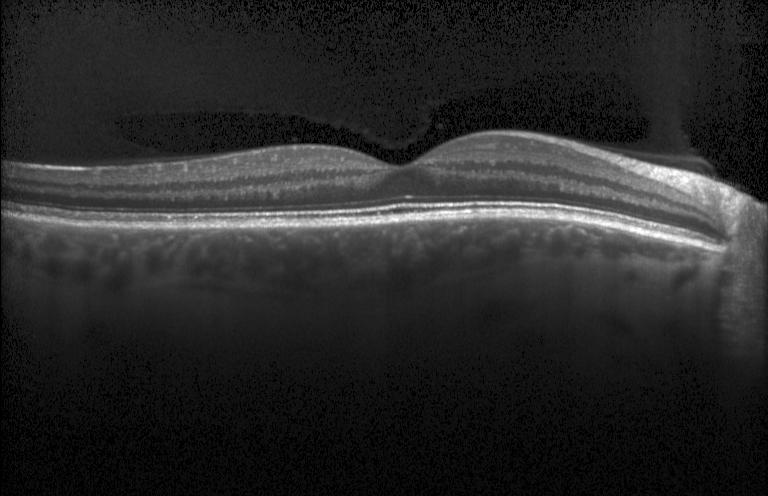 Spectral-domain optical coherence tomography. Optical coherence tomography scan. Acquired on a Heidelberg Spectralis. Macular scan.
The scan shows no choroidal neovascularization, diabetic macular edema, or drusen.